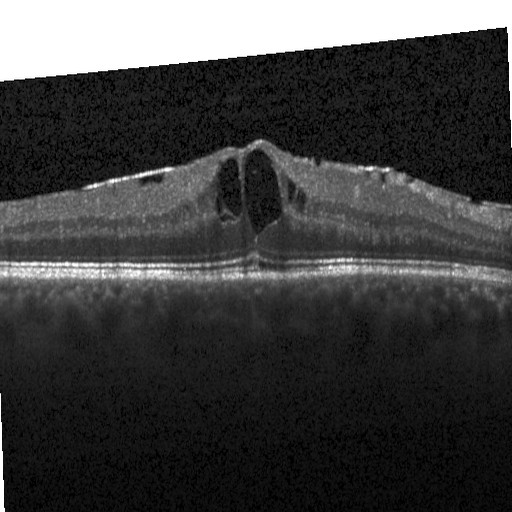
OCT line scan. Impression: DME.